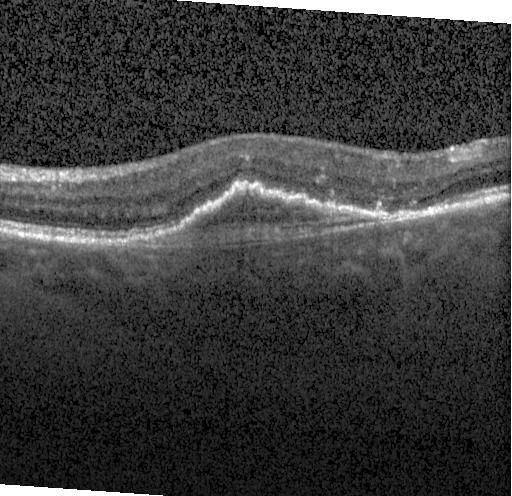

Fovea-centered; retinal OCT cross-section; spectral-domain optical coherence tomography. Impression: choroidal neovascularization (CNV).